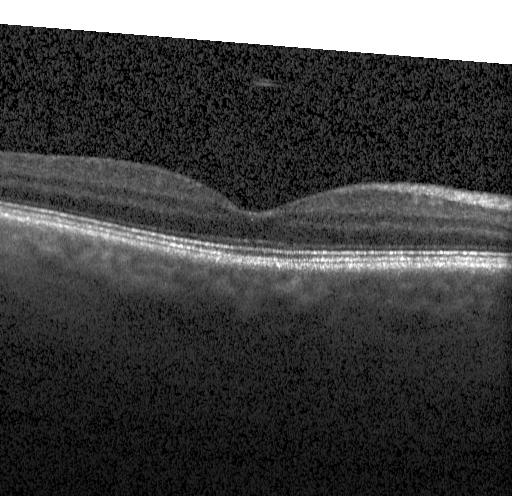
Retinal OCT B-scan — Finding: neither CNV, DME, nor drusen.